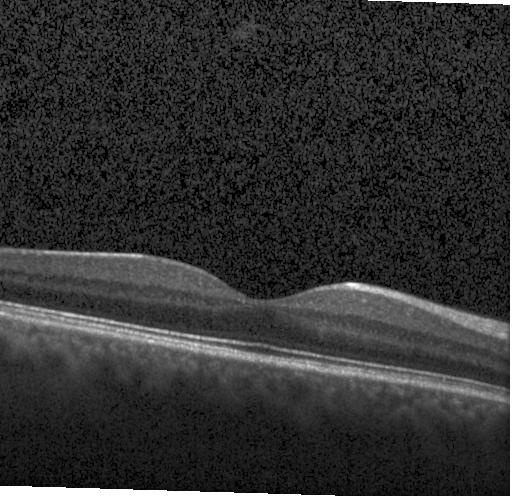

Acquired on a Heidelberg Spectralis · retinal OCT cross-section · spectral-domain optical coherence tomography — Finding: no CNV, no DME, and no drusen.